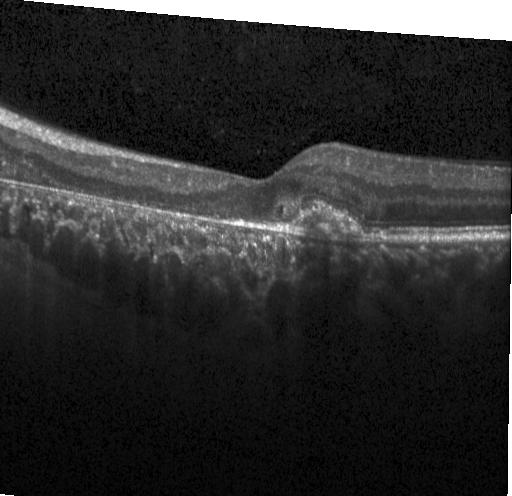
OCT finding: choroidal neovascularization.